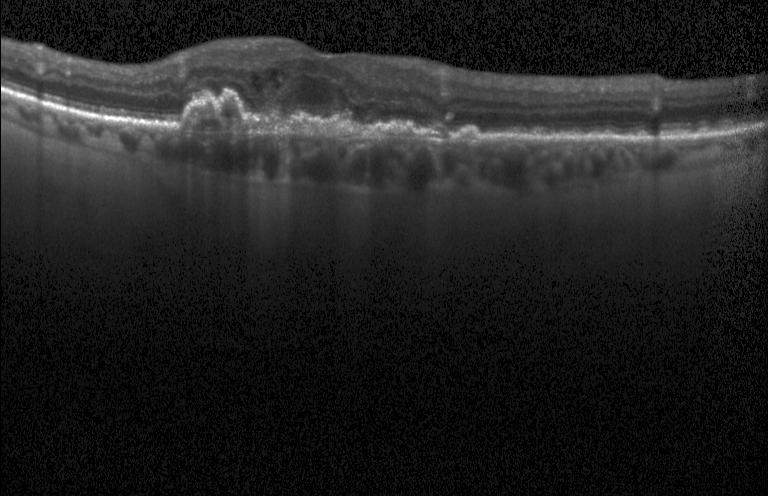 Finding: choroidal neovascularization (CNV).